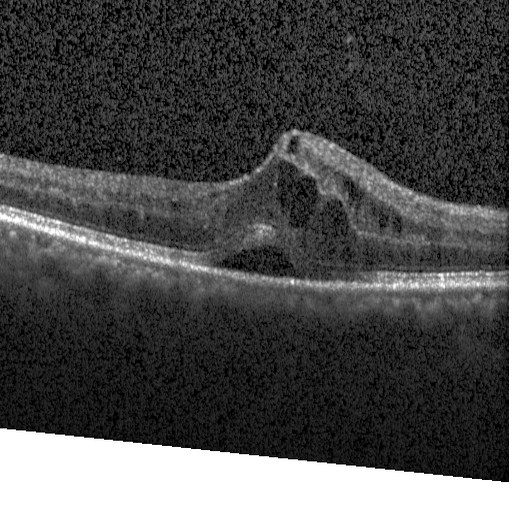

Impression: diabetic macular edema (DME).